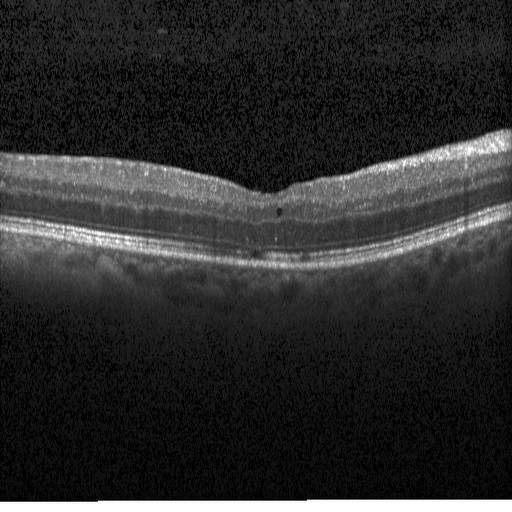 Diabetic macular edema.